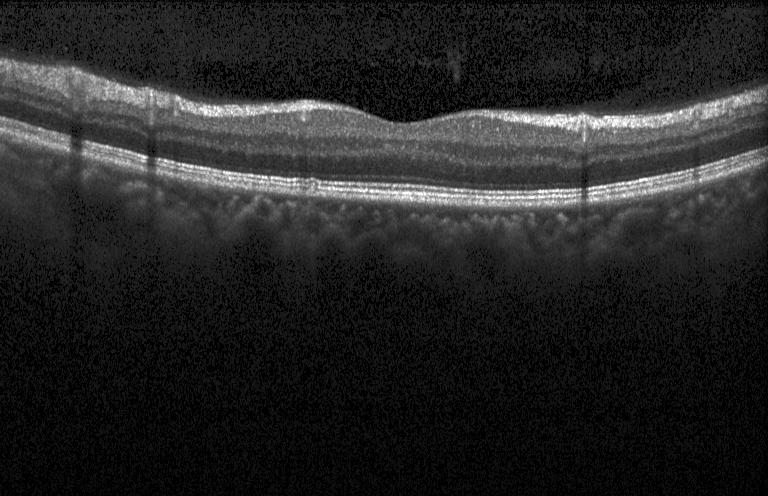

Through the macula · OCT B-scan · SD-OCT.
The scan shows no choroidal neovascularization, no diabetic macular edema, and no drusen.